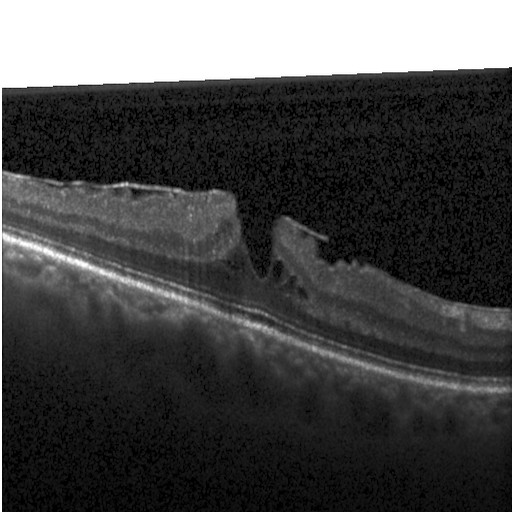
Heidelberg Spectralis OCT system · spectral-domain OCT · retinal OCT cross-section — Macular OCT: DME.